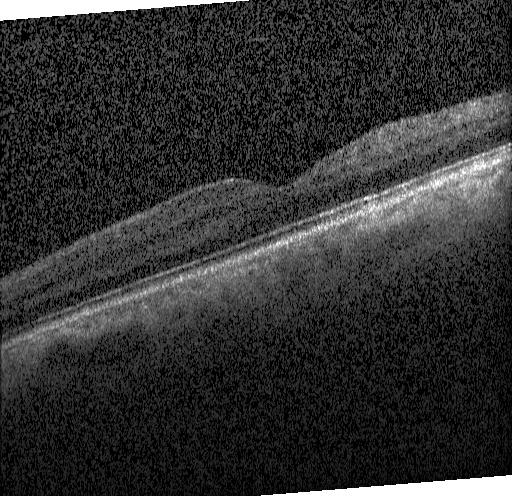
Acquired on a Heidelberg Spectralis · macular scan · OCT line scan — No evidence of CNV, DME, or drusen.